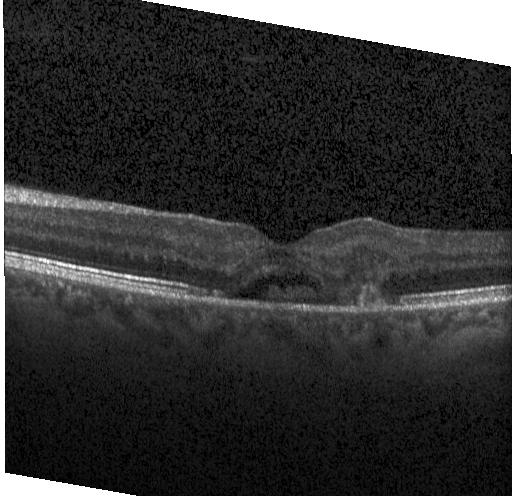 Horizontal scan through the fovea. Acquired on a Heidelberg Spectralis. Spectral-domain OCT. OCT B-scan — Finding: choroidal neovascularization.